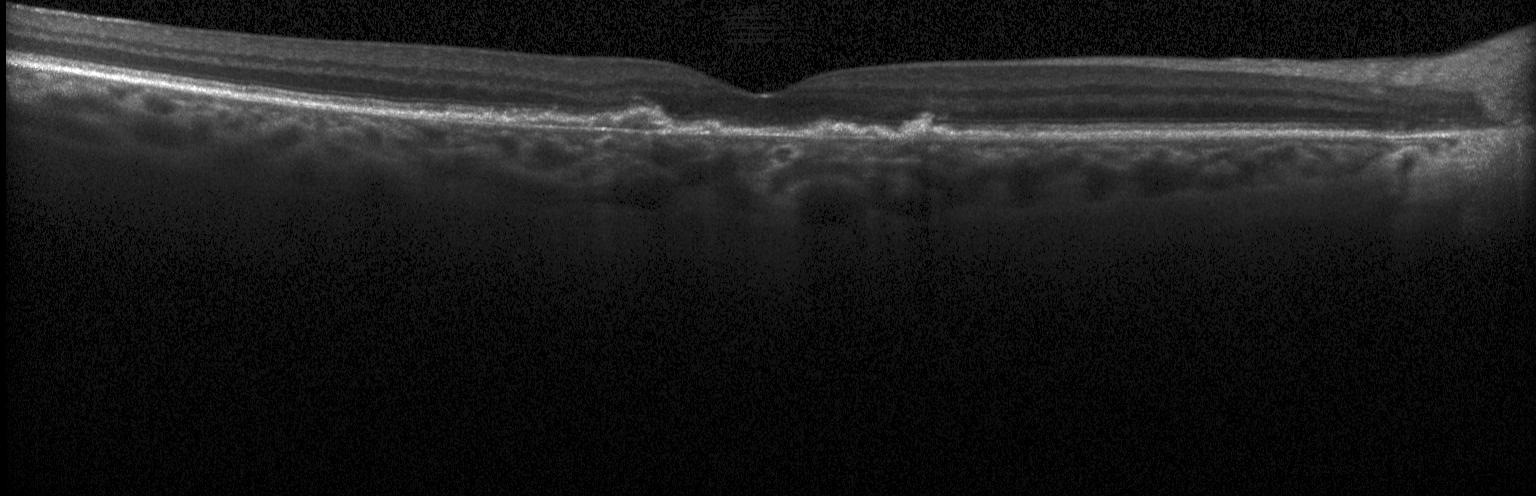 Retinal OCT cross-section. Horizontal scan through the fovea. Finding: choroidal neovascularization (CNV).